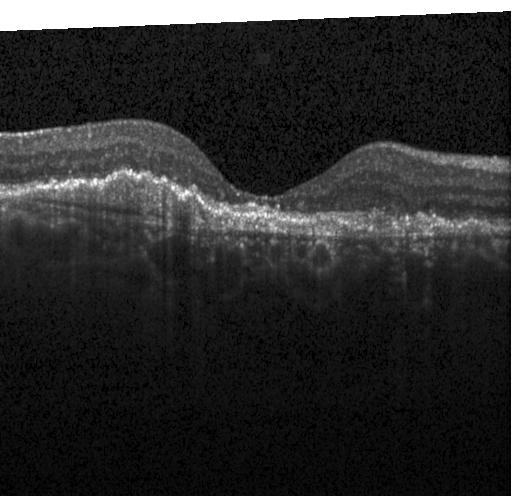
Retinal OCT cross-section.
Finding: a choroidal neovascular membrane.